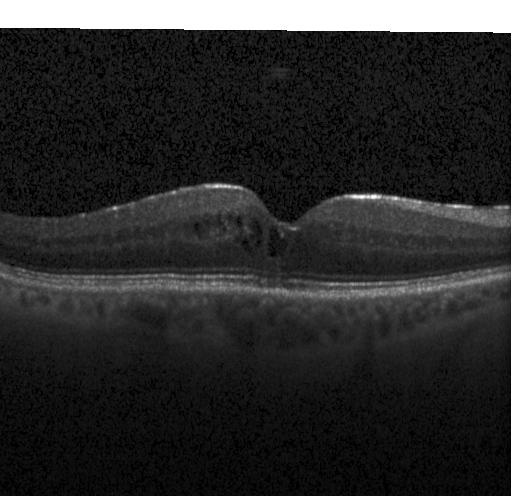 Impression: DME.